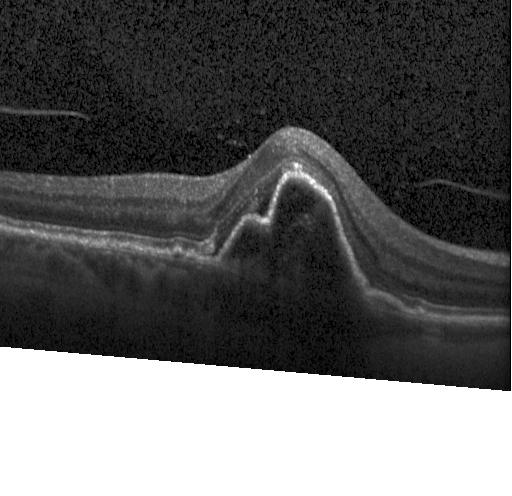 Fovea-centered; OCT B-scan; SD-OCT. Finding: choroidal neovascularization.